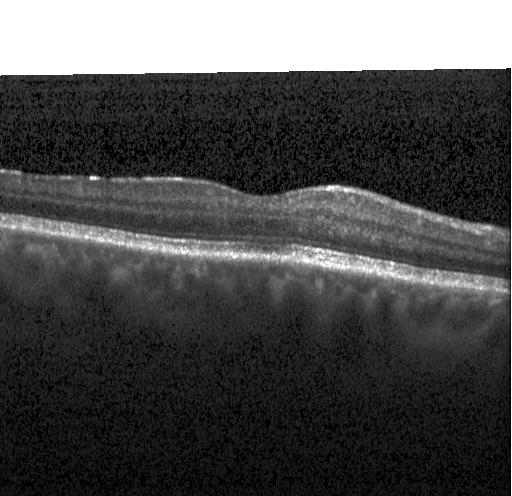
Spectral-domain OCT B-scan: no evidence of CNV, DME, or drusen.